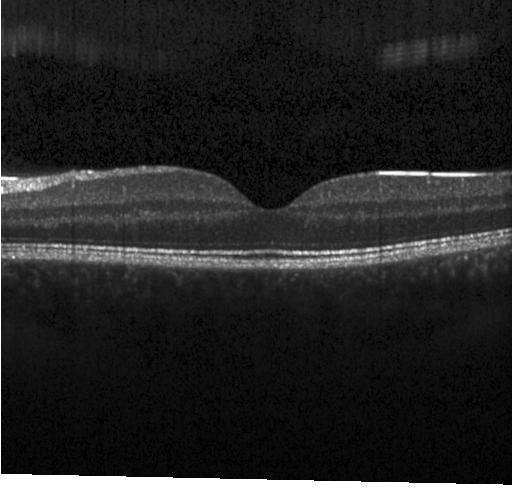

Retinal OCT B-scan, Heidelberg Spectralis OCT system — Impression: no choroidal neovascularization, no diabetic macular edema, and no drusen.